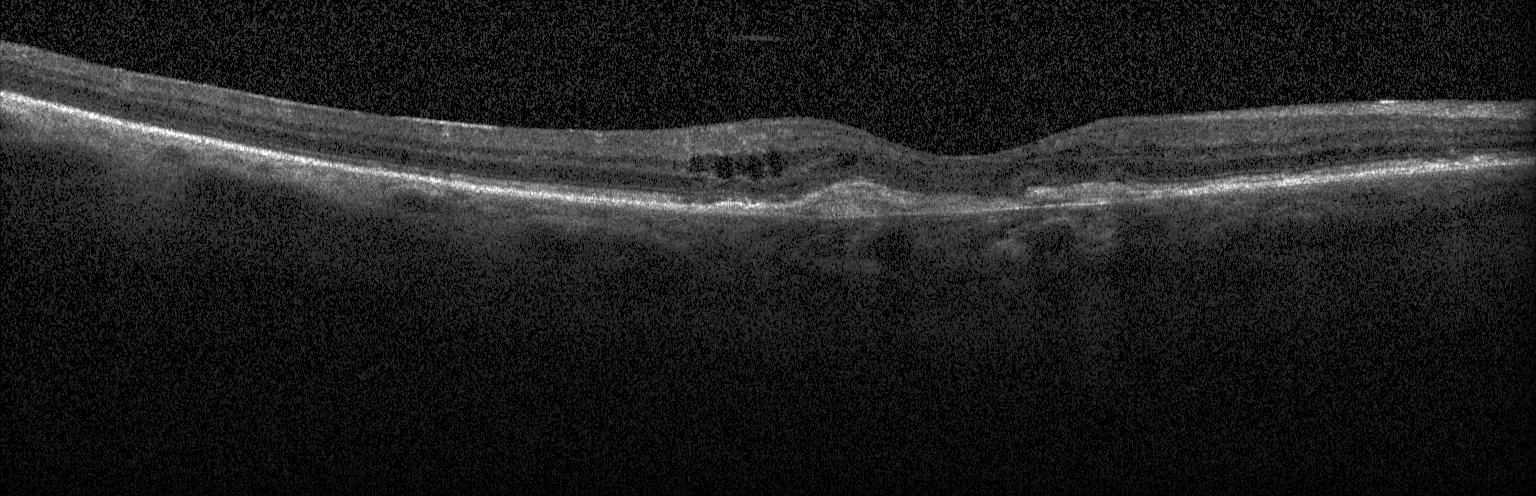
Retinal OCT B-scan. Assessment: CNV.